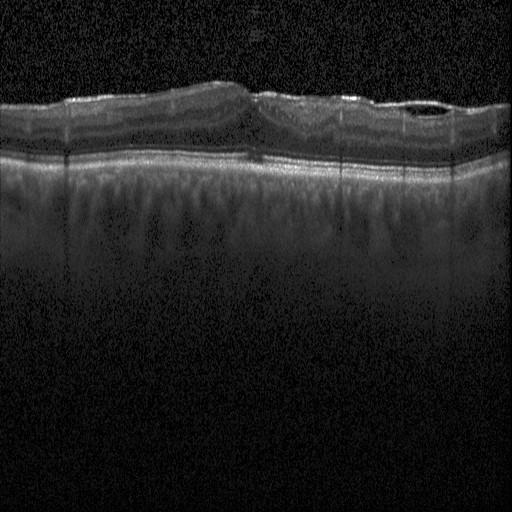

OCT B-scan
DME.